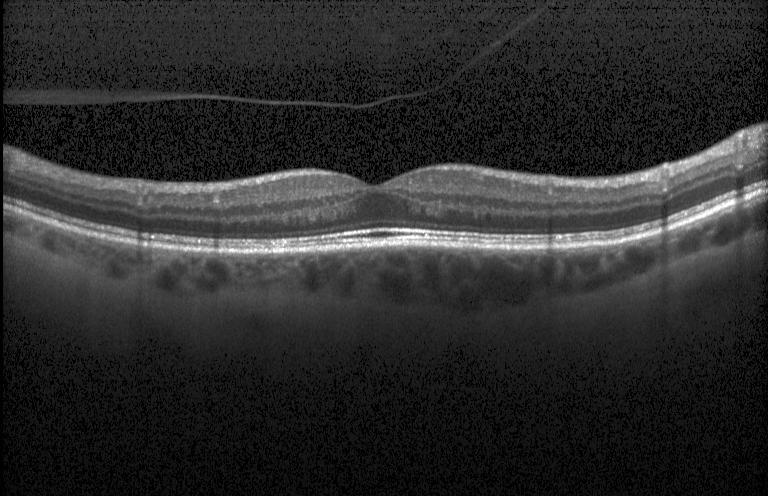

Diagnosis: no CNV, DME, or drusen.